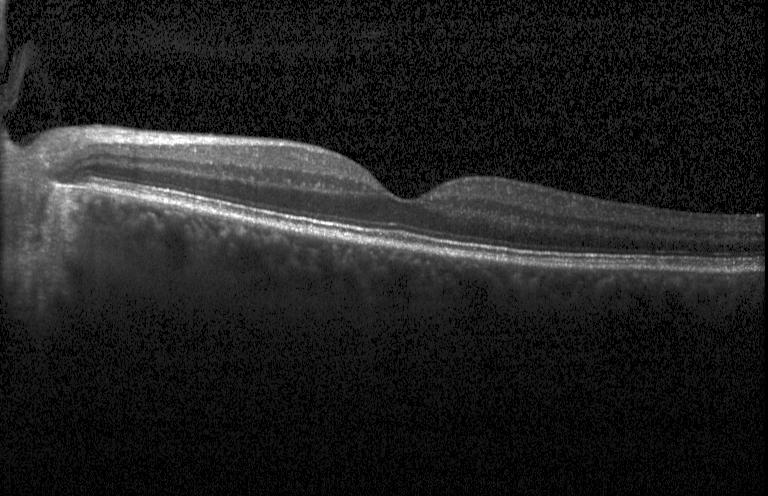
Diagnosis: neither choroidal neovascularization, diabetic macular edema, nor drusen.